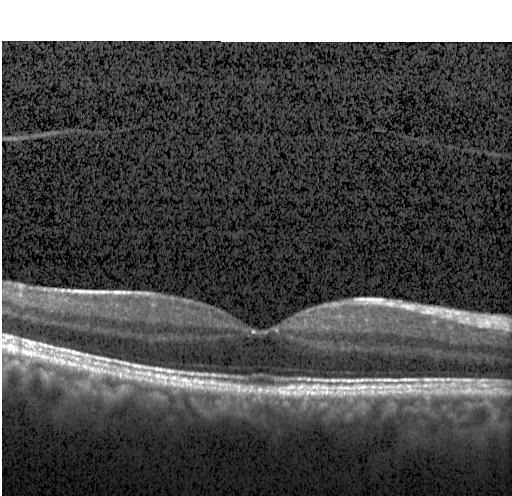

Retinal OCT cross-section — Assessment: no CNV, DME, or drusen.